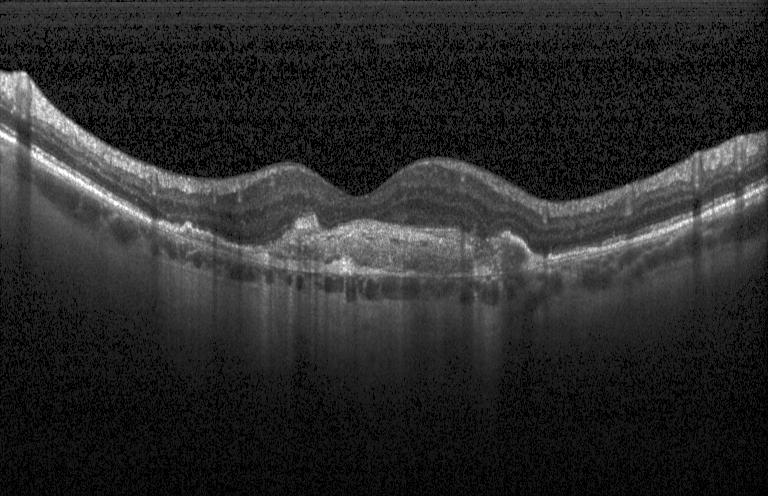 Macular OCT: choroidal neovascularization (CNV).